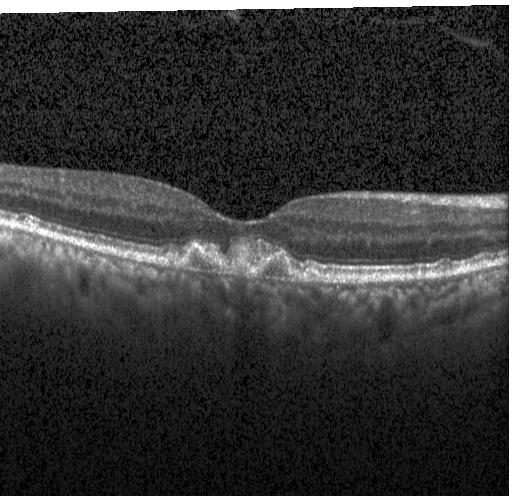 Optical coherence tomography scan · SD-OCT · horizontal scan through the fovea · Heidelberg Spectralis
Dx: a choroidal neovascular membrane.